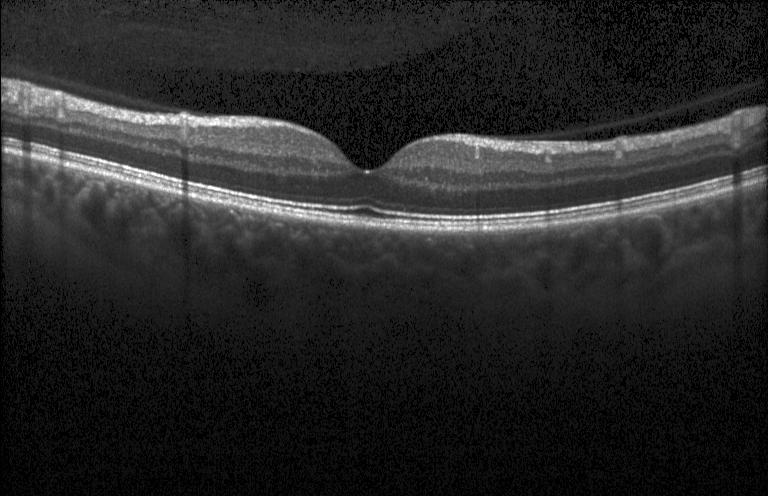

Optical coherence tomography scan — Neither choroidal neovascularization, diabetic macular edema, nor drusen.